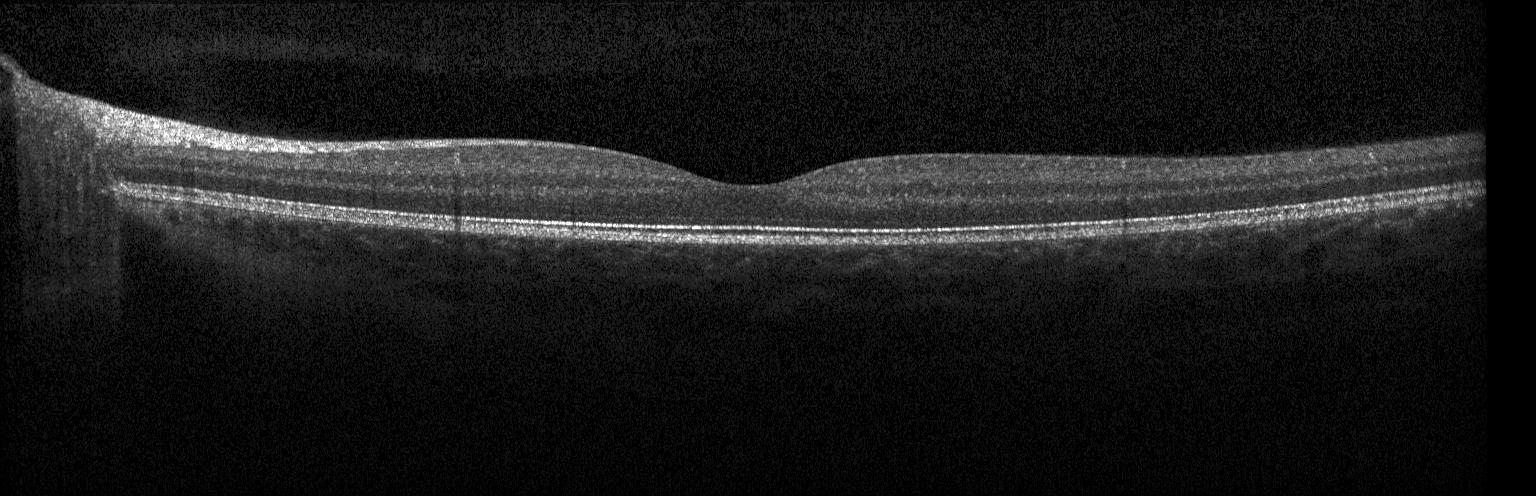 Macular OCT: no choroidal neovascularization, diabetic macular edema, or drusen.